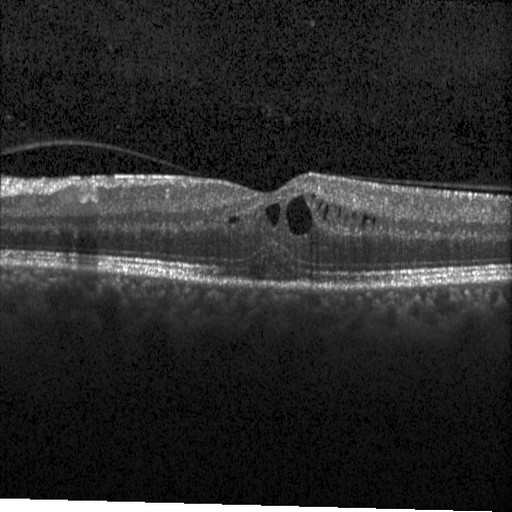 Impression: DME.